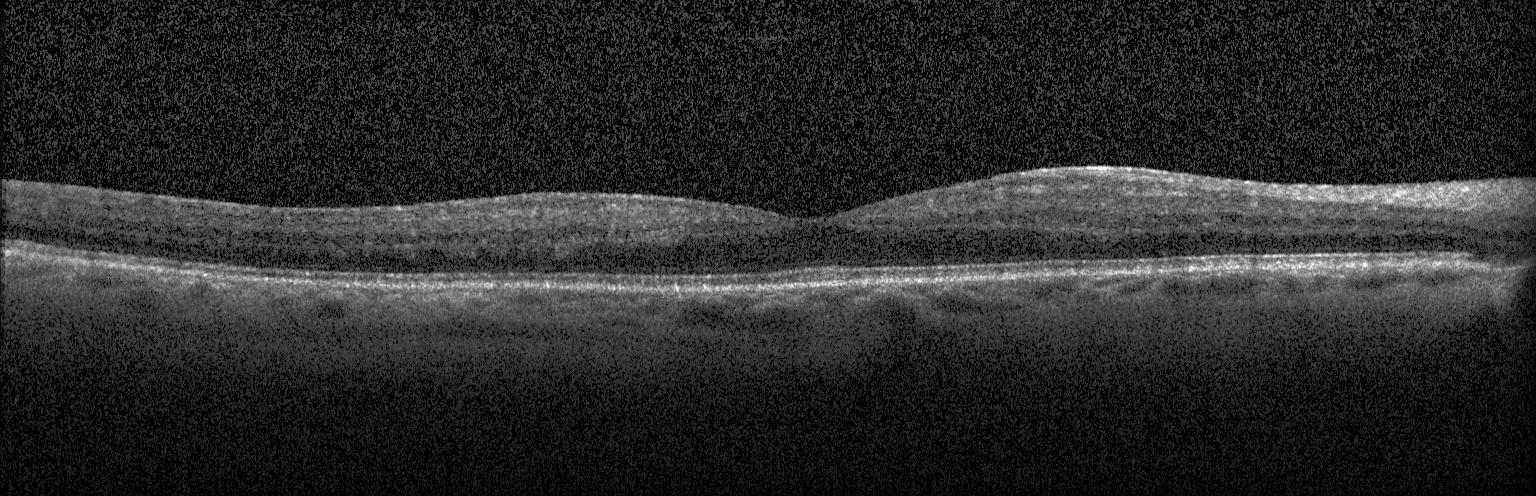 SD-OCT. Fovea-centered. OCT line scan — Finding: no choroidal neovascularization, diabetic macular edema, or drusen.